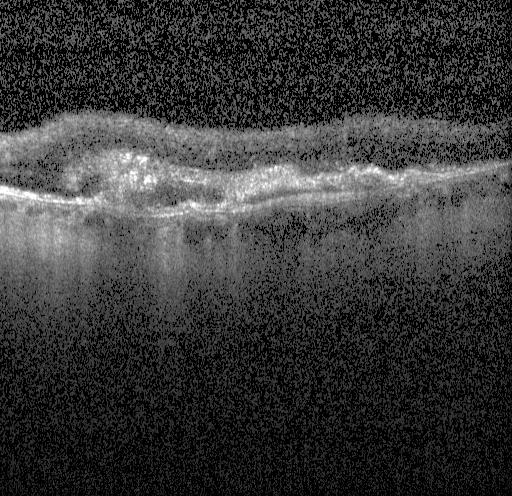 Optical coherence tomography scan — This B-scan demonstrates a choroidal neovascular membrane.